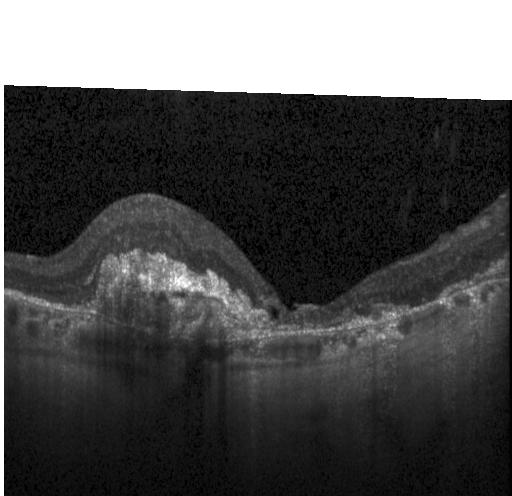

Instrument: Heidelberg Spectralis. SD-OCT. Centered on the fovea. OCT B-scan
The scan shows choroidal neovascularization (CNV).